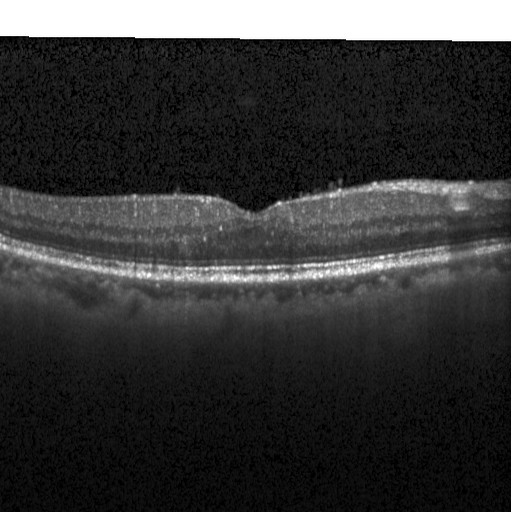

Macular OCT demonstrating diabetic macular edema.